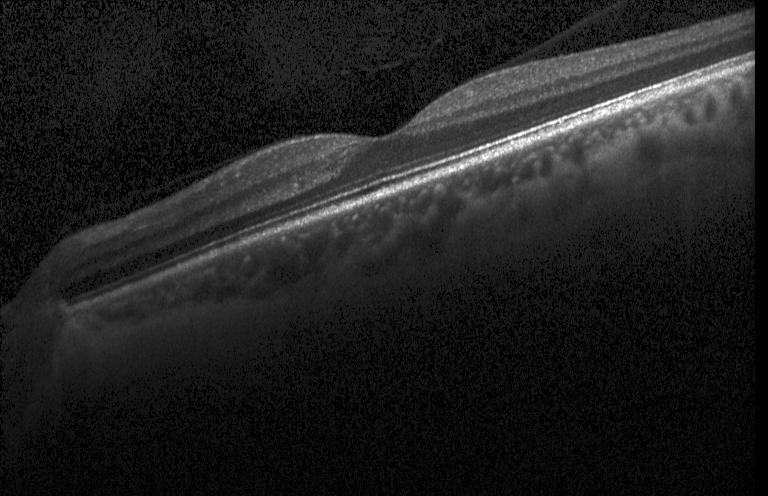

No CNV, no DME, and no drusen.